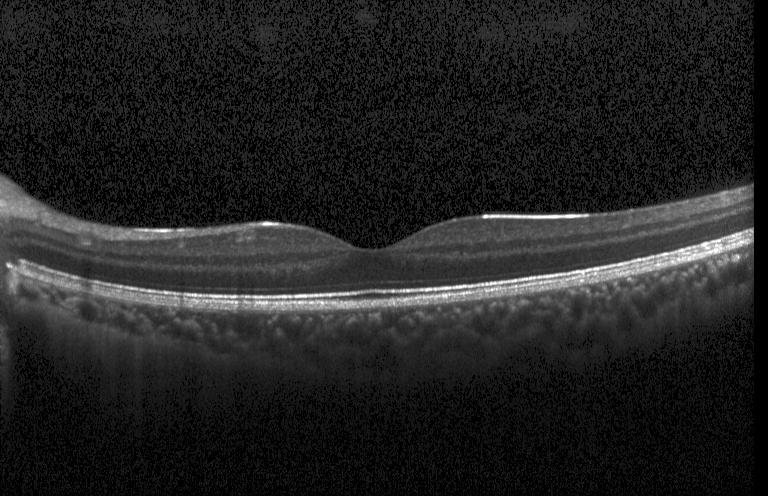

Retinal OCT cross-section; Heidelberg Spectralis.
Diagnosis: no choroidal neovascularization, diabetic macular edema, or drusen.